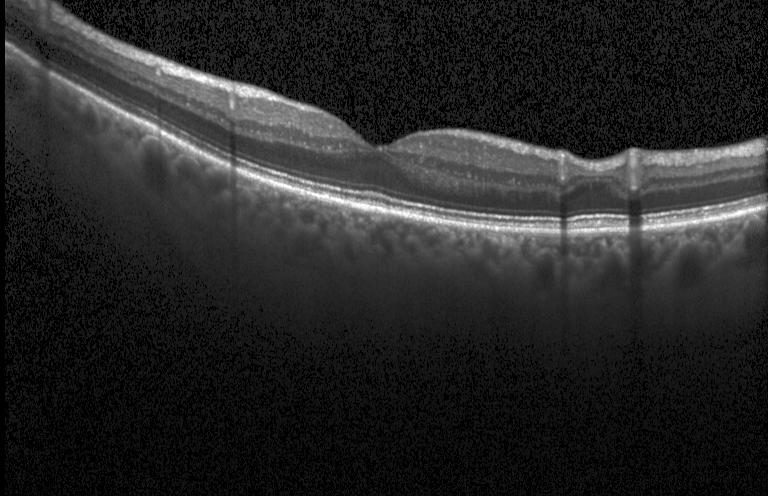

Retinal OCT cross-section. Heidelberg Spectralis OCT system. Through the macula
This B-scan demonstrates neither choroidal neovascularization, diabetic macular edema, nor drusen.